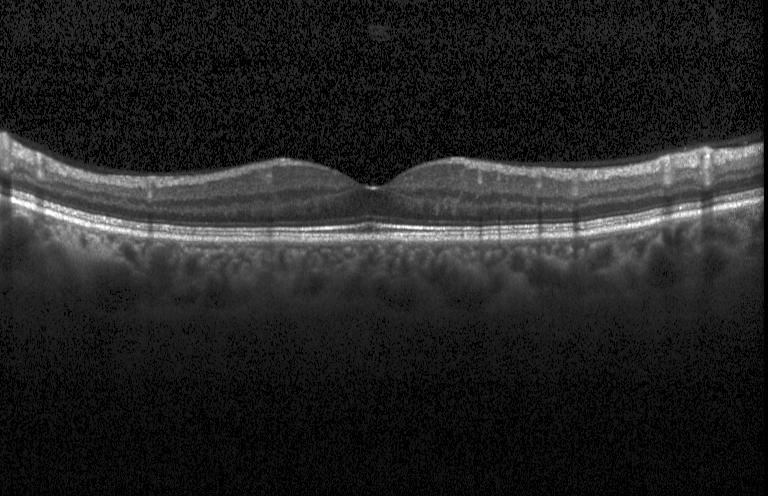
Macular OCT: neither choroidal neovascularization, diabetic macular edema, nor drusen.